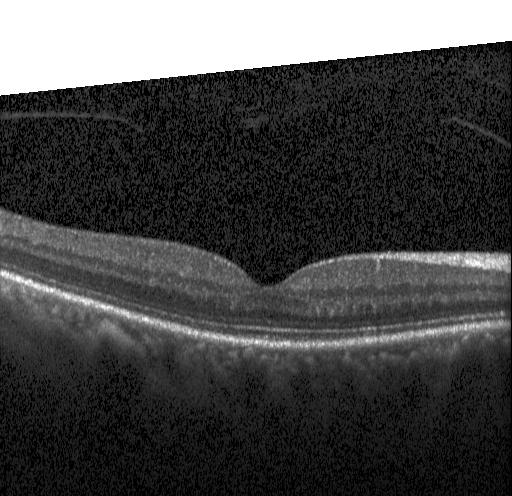

Heidelberg Spectralis OCT system. Fovea-centered. Spectral-domain OCT. Optical coherence tomography scan. Macular OCT: neither choroidal neovascularization, diabetic macular edema, nor drusen.